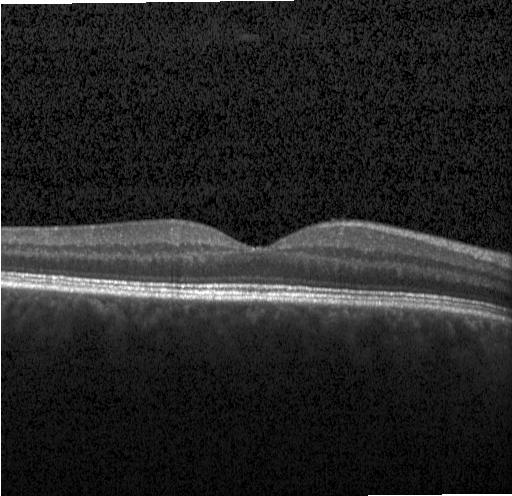
Heidelberg Spectralis, spectral-domain optical coherence tomography, retinal OCT cross-section. Assessment: no choroidal neovascularization, no diabetic macular edema, and no drusen.